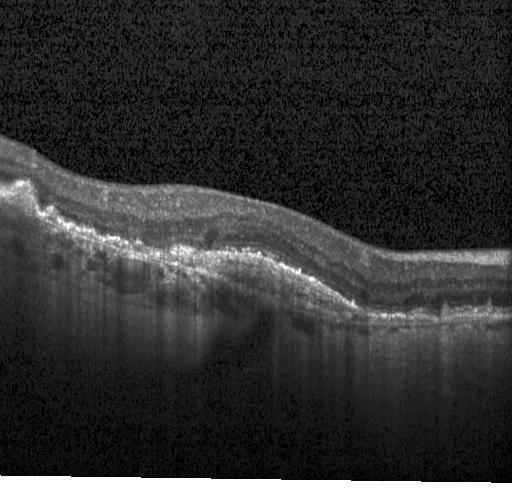

Optical coherence tomography B-scan
Macular OCT: a choroidal neovascular membrane.